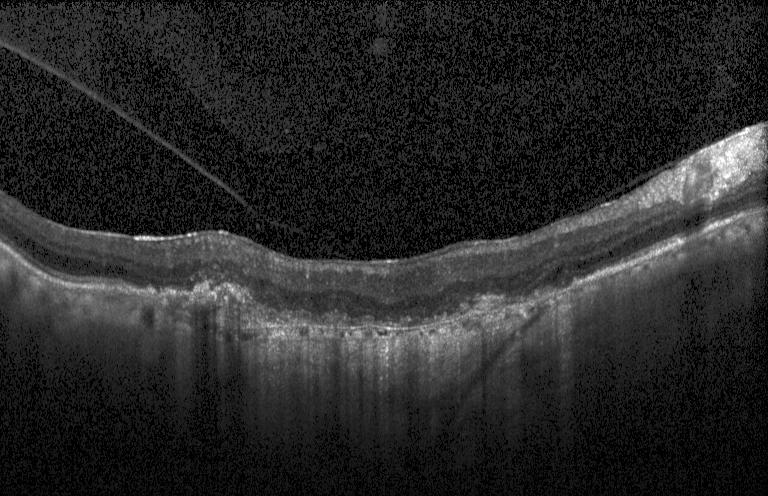 Optical coherence tomography B-scan · acquired on a Heidelberg Spectralis · spectral-domain optical coherence tomography · centered on the fovea
Finding: choroidal neovascularization (CNV).